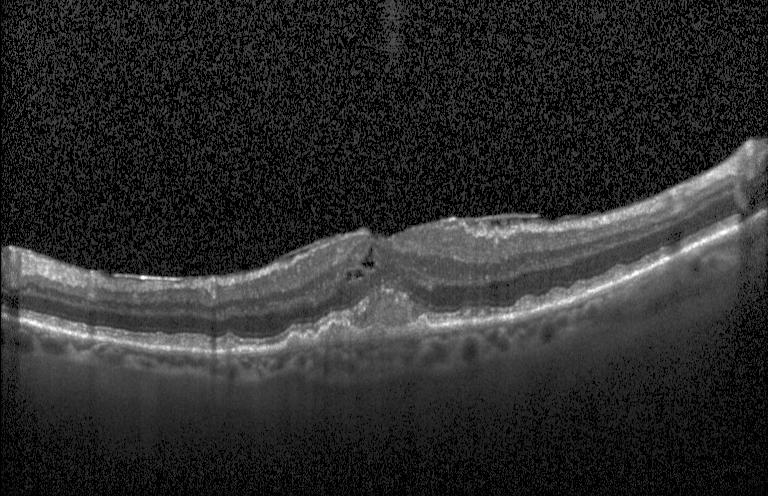

Impression: CNV.